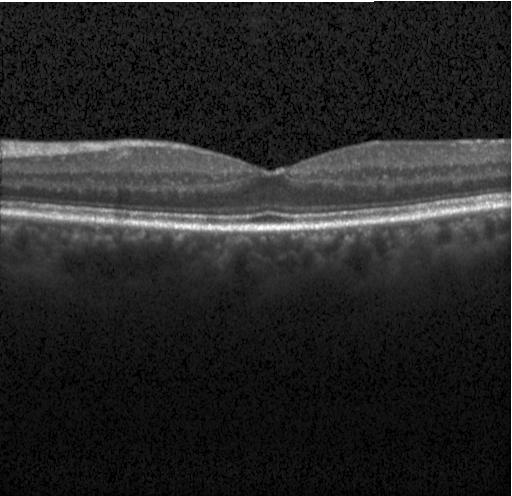
OCT B-scan showing no evidence of choroidal neovascularization, diabetic macular edema, or drusen.